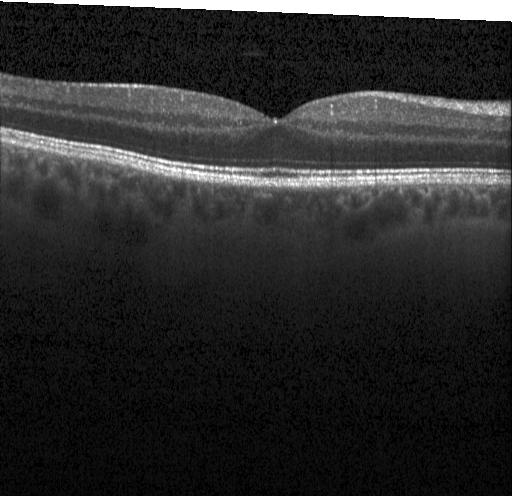 Retinal OCT cross-section showing no choroidal neovascularization, diabetic macular edema, or drusen.